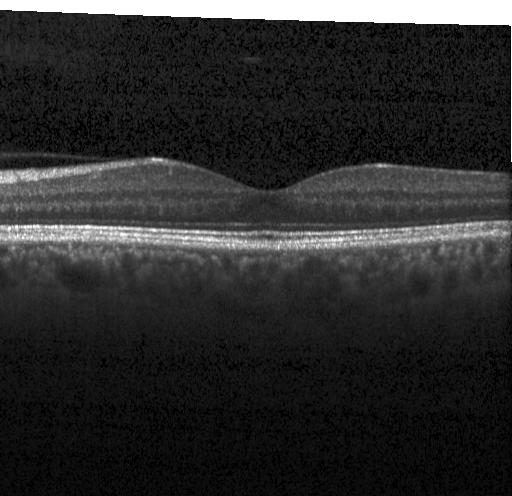

Fovea-centered · spectral-domain optical coherence tomography · retinal OCT B-scan · Heidelberg Spectralis.
This B-scan demonstrates neither choroidal neovascularization, diabetic macular edema, nor drusen.